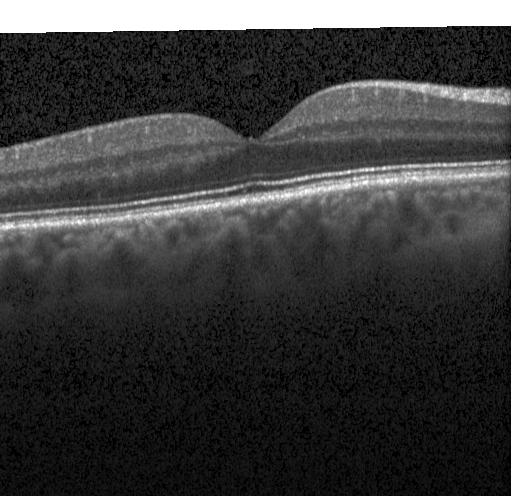
Assessment: neither CNV, DME, nor drusen.